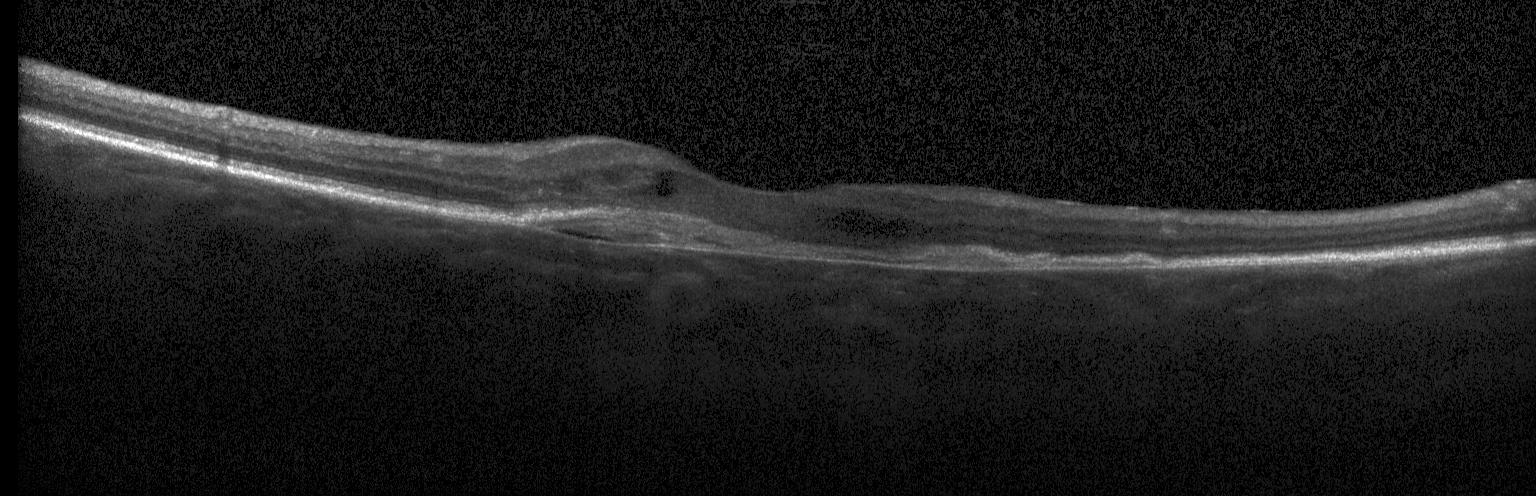

Finding: choroidal neovascularization.